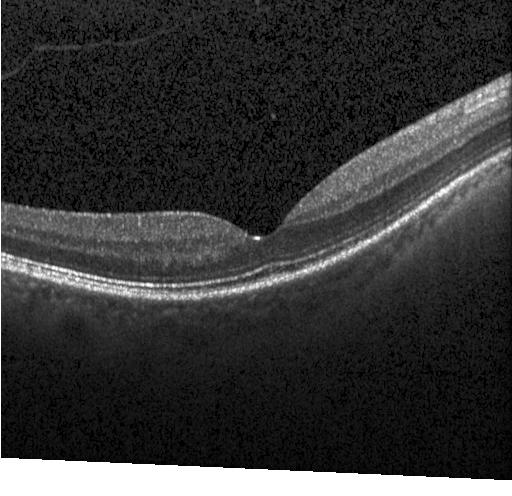 Finding: no evidence of choroidal neovascularization, diabetic macular edema, or drusen.